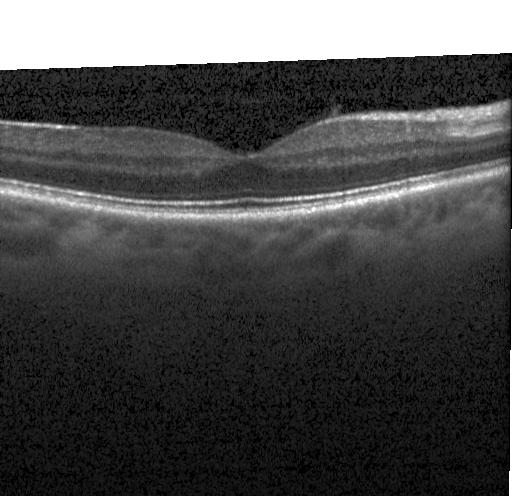

Retinal OCT B-scan — Assessment: neither CNV, DME, nor drusen.